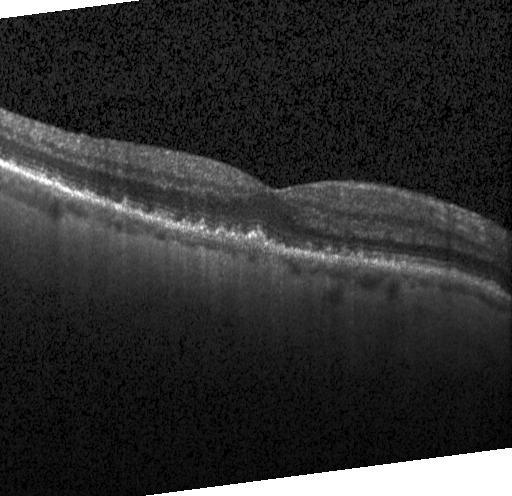

Dx: drusen.